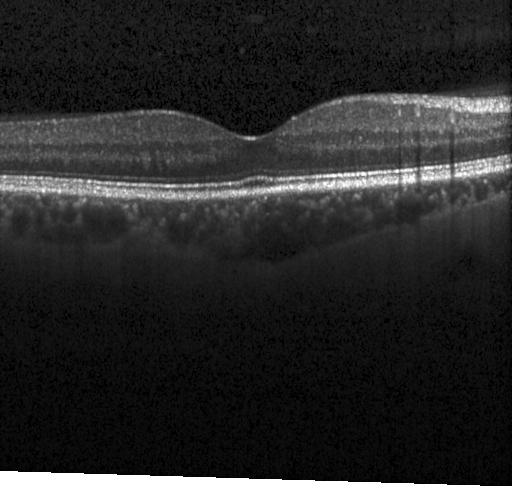 Retinal OCT cross-section showing neither choroidal neovascularization, diabetic macular edema, nor drusen.